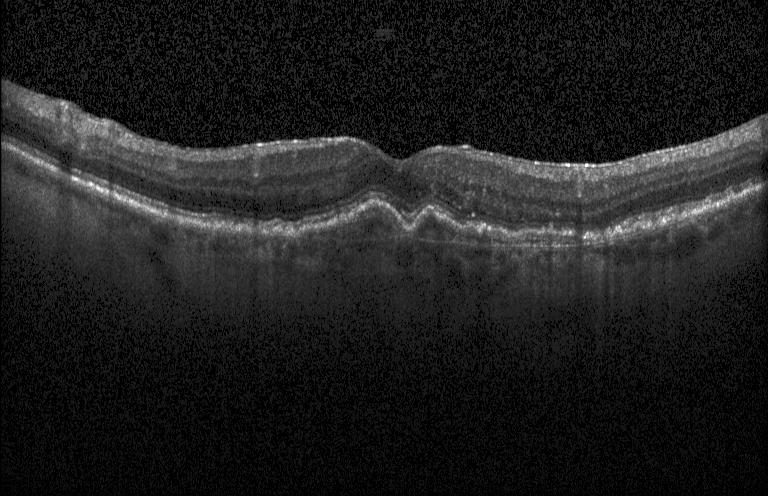 Optical coherence tomography B-scan, macular scan, Heidelberg Spectralis — The scan shows a choroidal neovascular membrane.